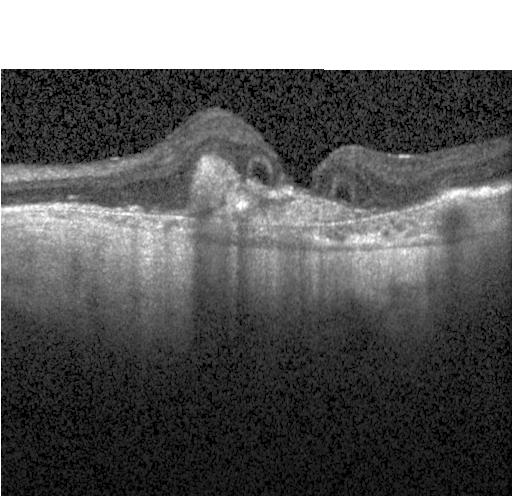 Spectral-domain optical coherence tomography. Through the macula. OCT B-scan. Instrument: Heidelberg Spectralis
Finding: CNV.